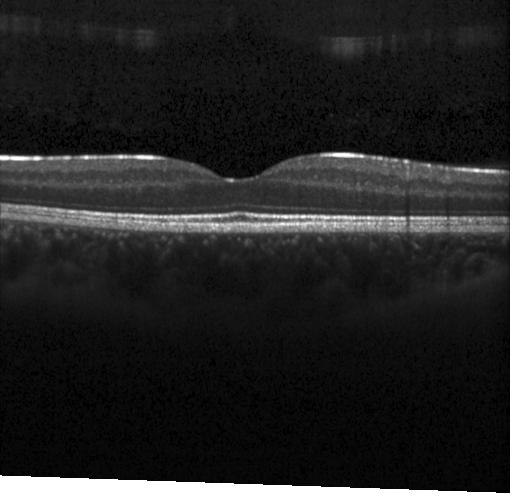
Diagnosis: no choroidal neovascularization, no diabetic macular edema, and no drusen.